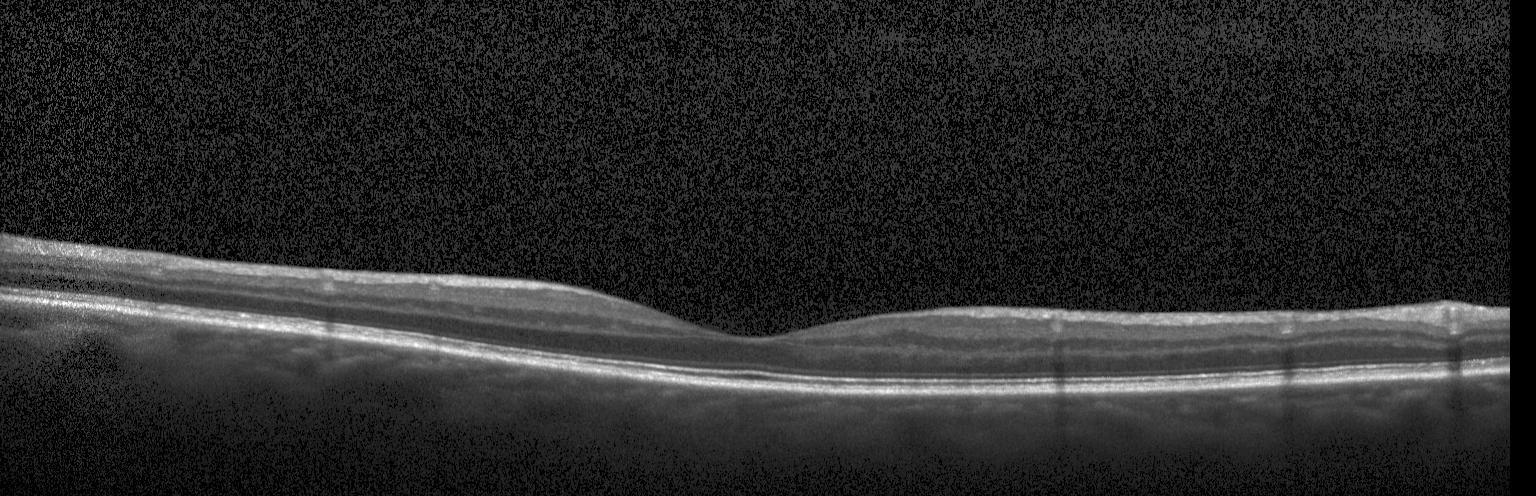

OCT line scan. Horizontal scan through the fovea
This B-scan demonstrates no choroidal neovascularization, no diabetic macular edema, and no drusen.